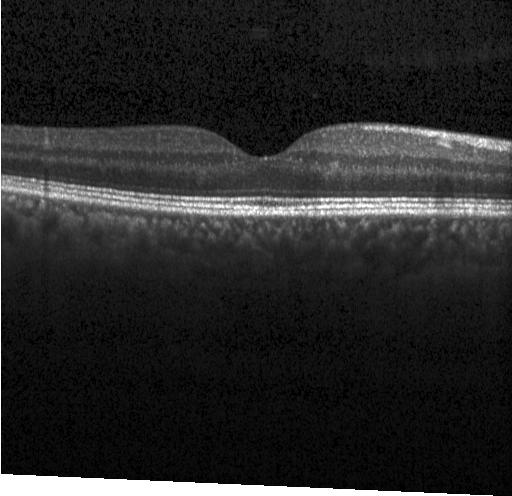
OCT B-scan showing no CNV, DME, or drusen.